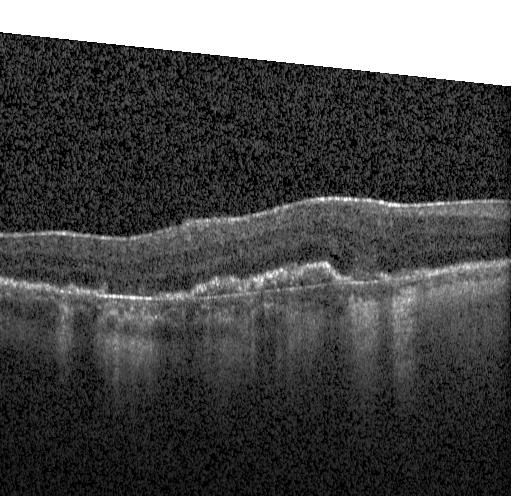 Macular scan · spectral-domain OCT · instrument: Heidelberg Spectralis · optical coherence tomography scan.
Macular OCT: choroidal neovascularization (CNV).